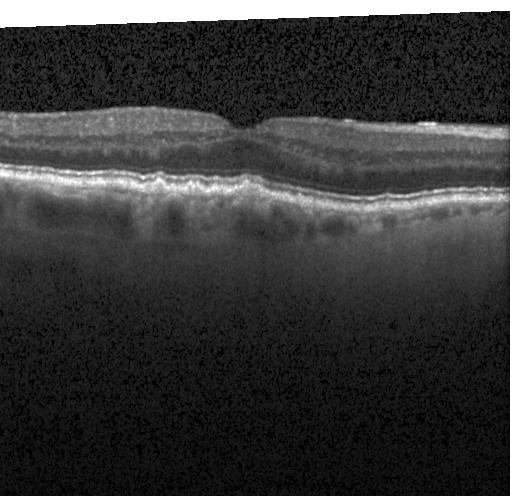

Diagnosis: sub-RPE drusenoid deposits.